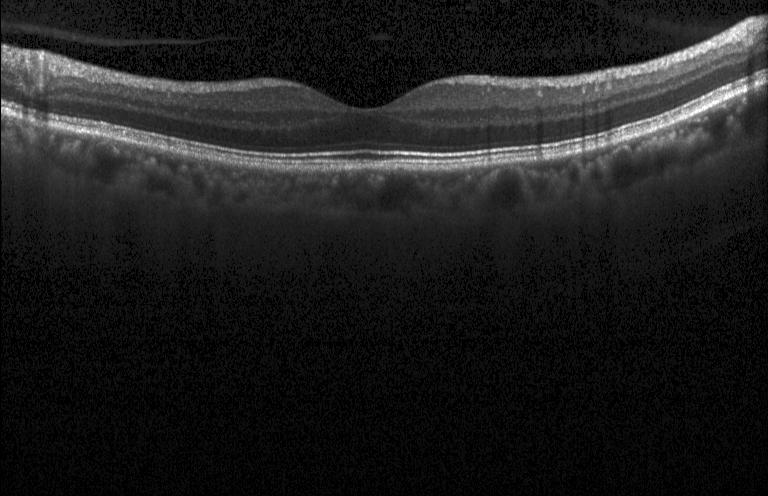
OCT line scan, horizontal scan through the fovea — Impression: no choroidal neovascularization, diabetic macular edema, or drusen.